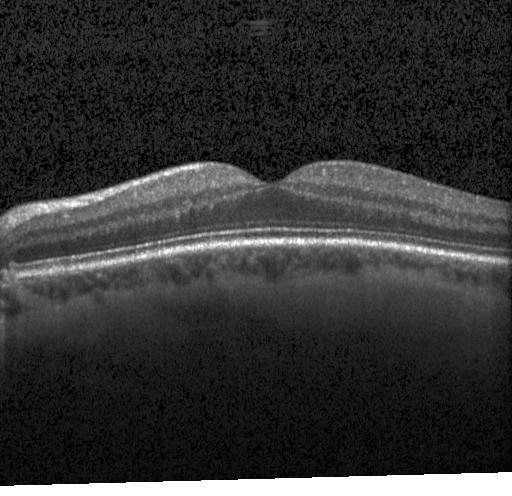
Retinal OCT cross-section showing neither choroidal neovascularization, diabetic macular edema, nor drusen.